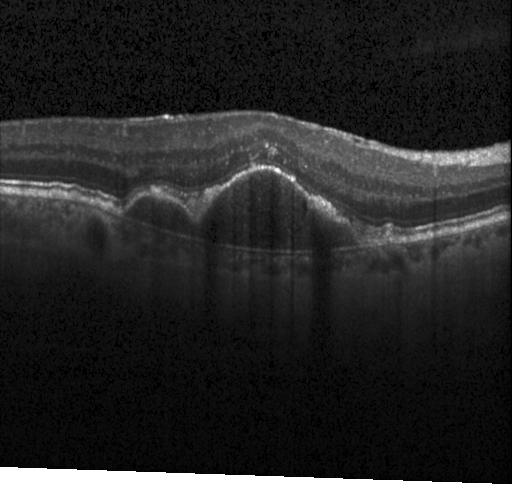

OCT B-scan, through the macula — Macular OCT: choroidal neovascularization.